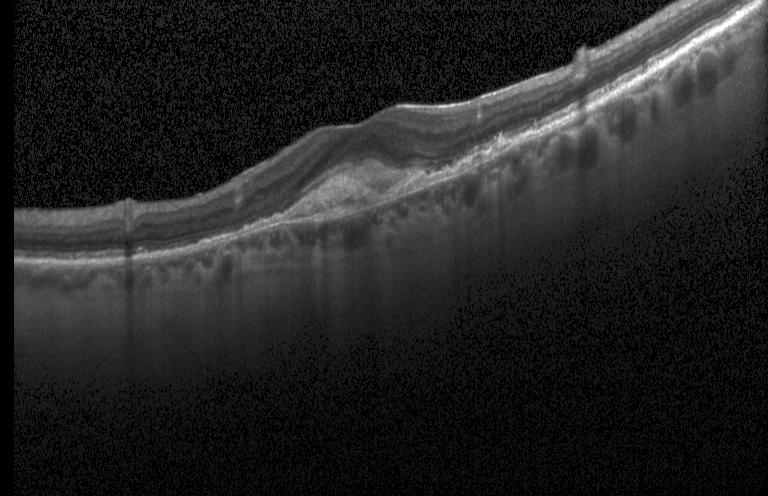
Optical coherence tomography scan. The scan shows a choroidal neovascular membrane.